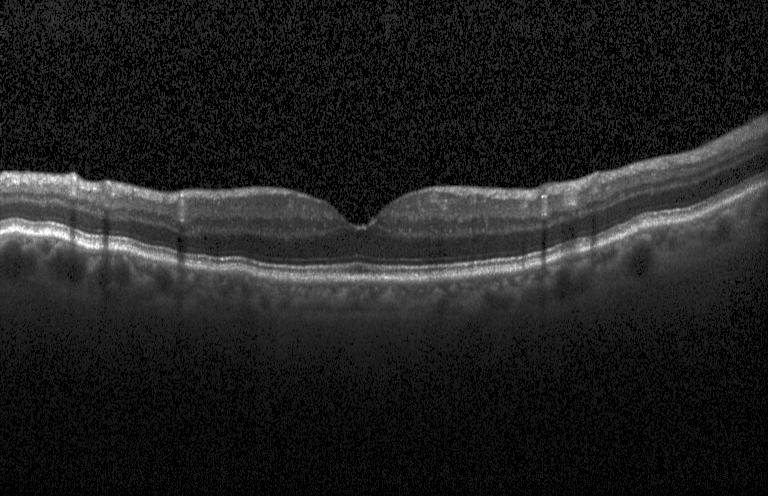

OCT scan showing neither choroidal neovascularization, diabetic macular edema, nor drusen.